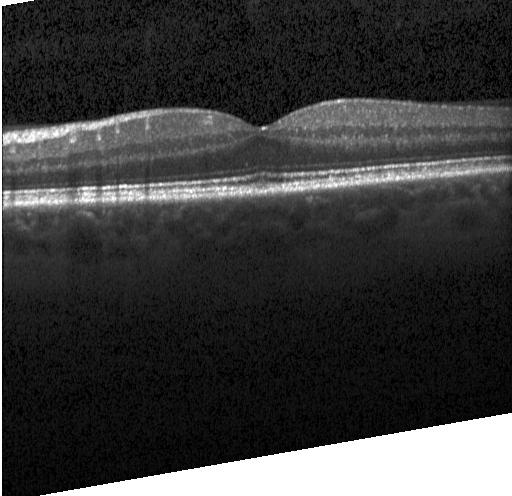 Finding: no evidence of CNV, DME, or drusen.